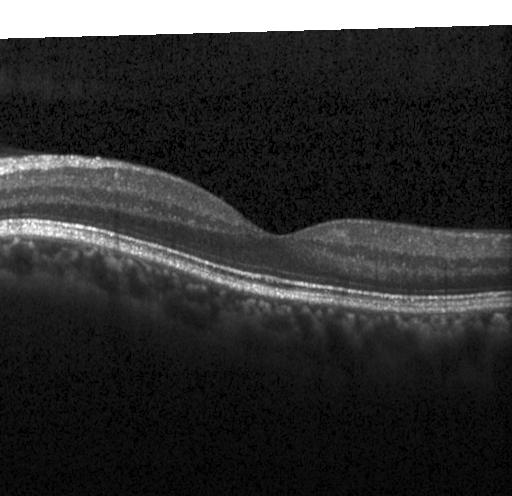

Retinal OCT cross-section — No choroidal neovascularization, diabetic macular edema, or drusen.